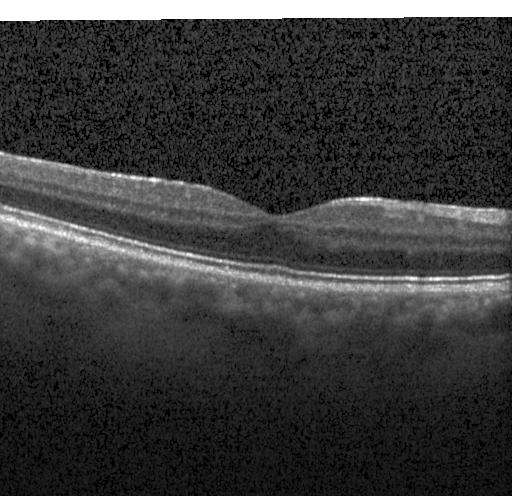 OCT B-scan · spectral-domain OCT · instrument: Heidelberg Spectralis · through the macula
This B-scan demonstrates no CNV, DME, or drusen.